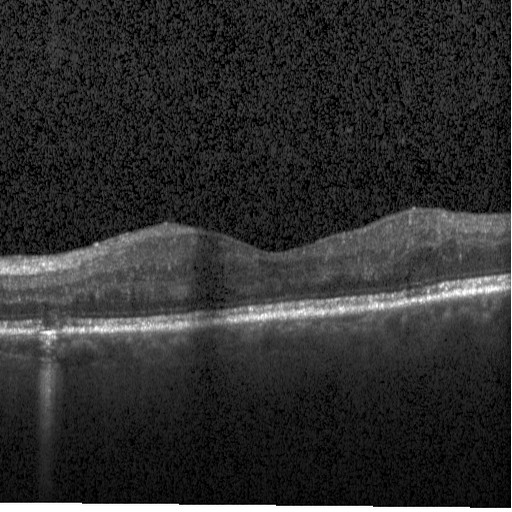 Through the macula; retinal OCT B-scan; instrument: Heidelberg Spectralis; spectral-domain OCT
This B-scan demonstrates diabetic macular edema.